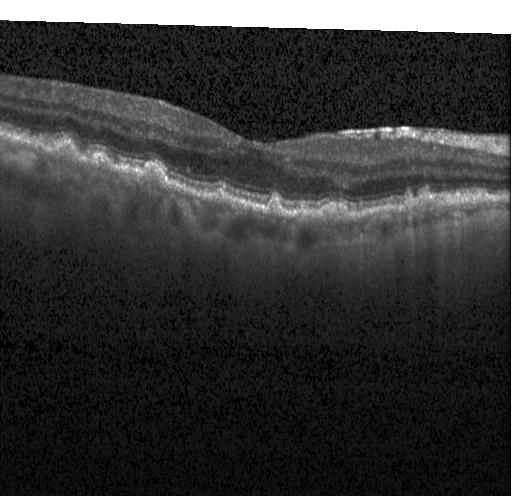
OCT scan showing sub-RPE drusenoid deposits.